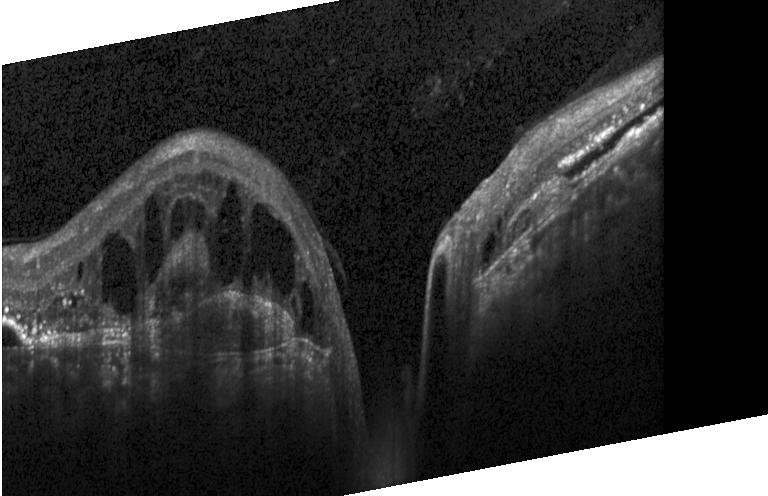
Spectral-domain OCT B-scan: a choroidal neovascular membrane.